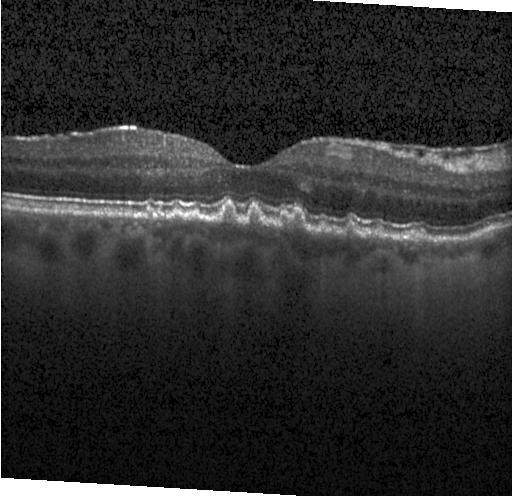 Finding: multiple drusen.